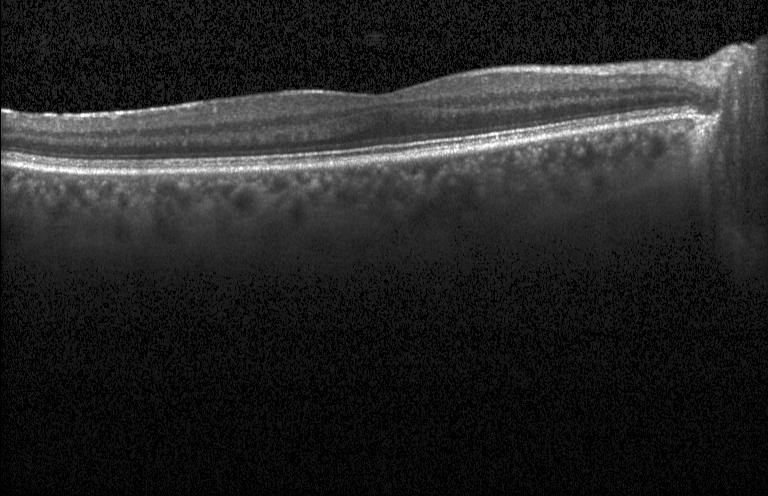

OCT B-scan, SD-OCT.
No evidence of choroidal neovascularization, diabetic macular edema, or drusen.